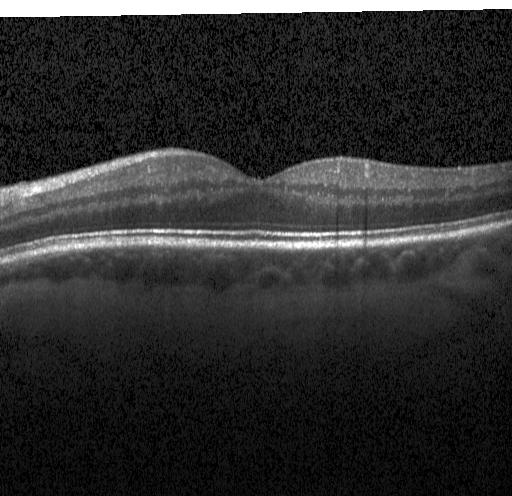 OCT line scan; through the macula
Impression: no evidence of CNV, DME, or drusen.